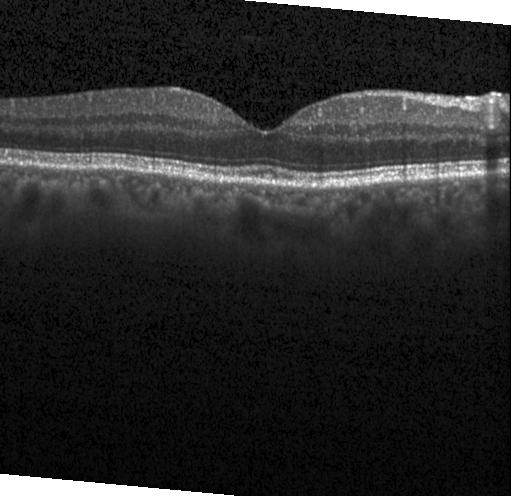
Impression: no choroidal neovascularization, diabetic macular edema, or drusen.